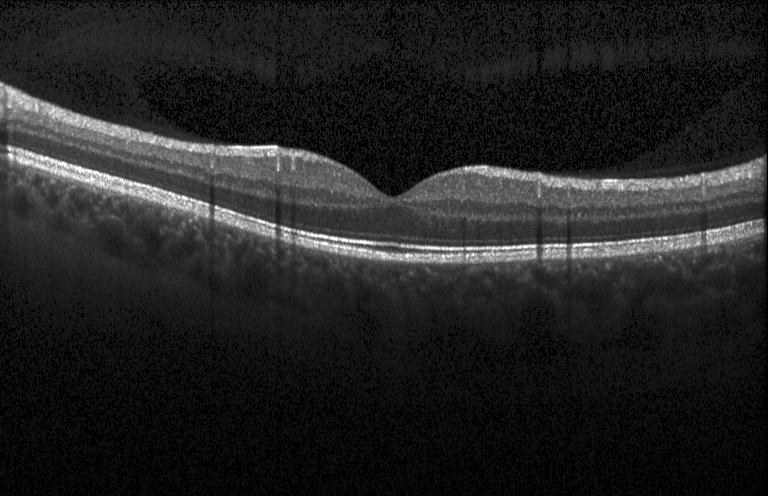
Retinal OCT cross-section, Heidelberg Spectralis OCT system, horizontal scan through the fovea, spectral-domain optical coherence tomography
Diagnosis: neither CNV, DME, nor drusen.